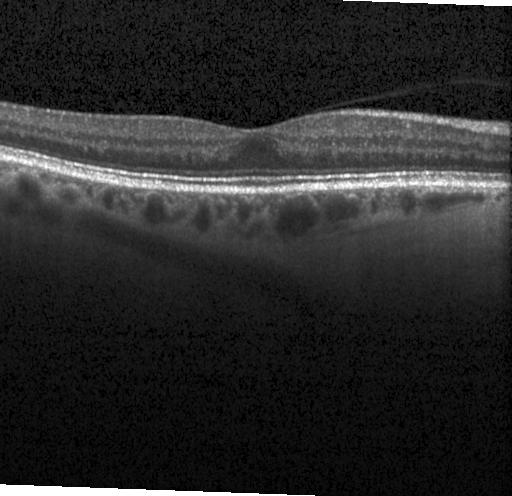
Spectral-domain optical coherence tomography; acquired on a Heidelberg Spectralis; retinal OCT B-scan. Impression: no choroidal neovascularization, diabetic macular edema, or drusen.